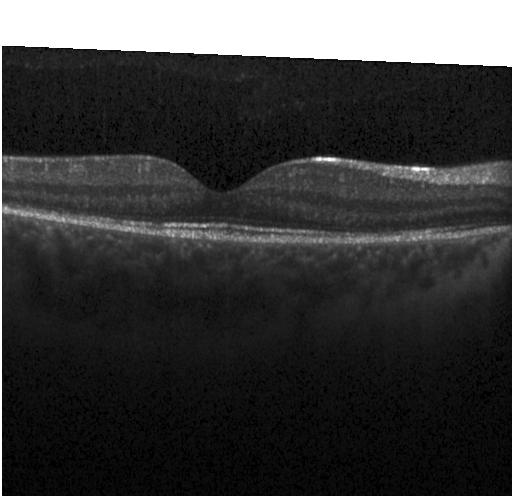
Optical coherence tomography scan. Assessment: no choroidal neovascularization, no diabetic macular edema, and no drusen.